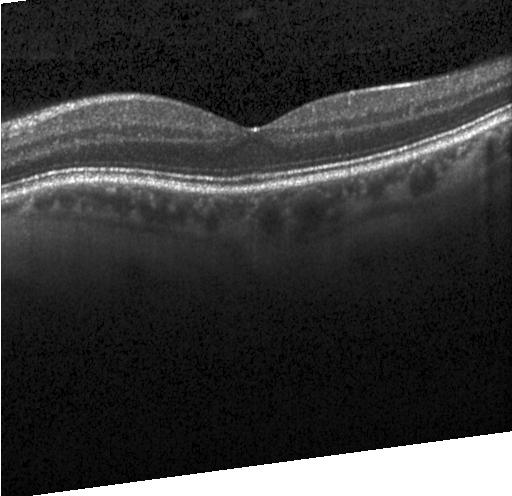 The scan shows no choroidal neovascularization, diabetic macular edema, or drusen.